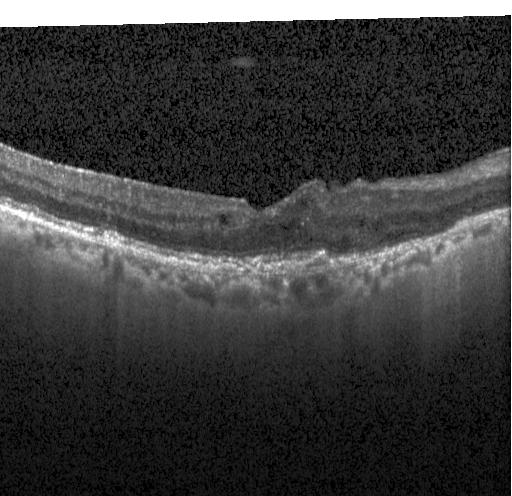
Impression: a choroidal neovascular membrane.